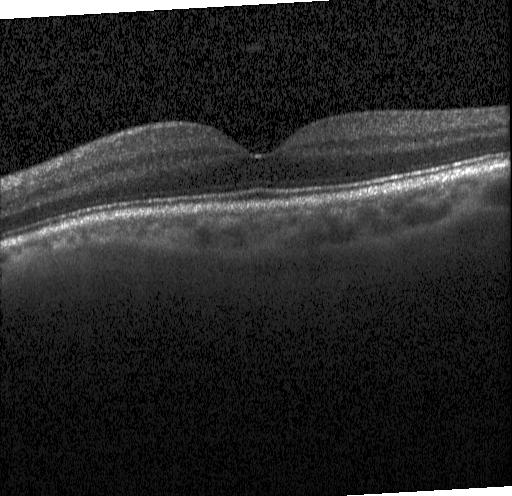 Impression: no evidence of choroidal neovascularization, diabetic macular edema, or drusen.